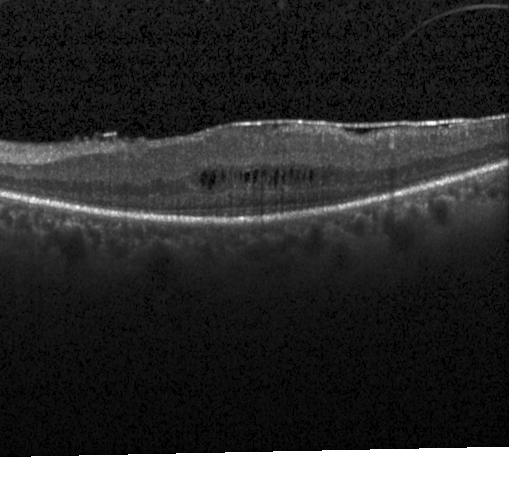

Spectral-domain OCT, through the macula, Heidelberg Spectralis OCT system, OCT line scan — Macular OCT: diabetic macular edema (DME).